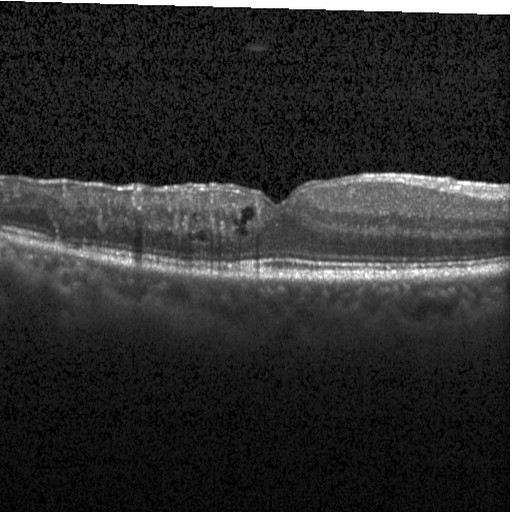 Optical coherence tomography scan. SD-OCT. Instrument: Heidelberg Spectralis. Through the macula — Diagnosis: diabetic macular edema (DME).